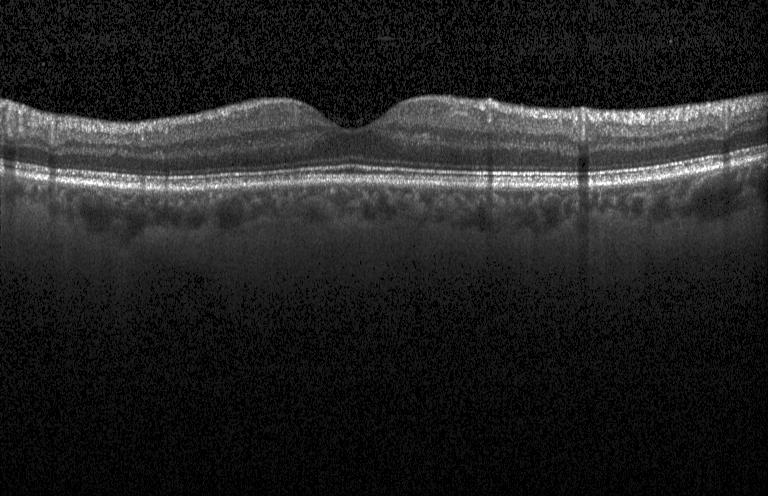 No evidence of CNV, DME, or drusen.